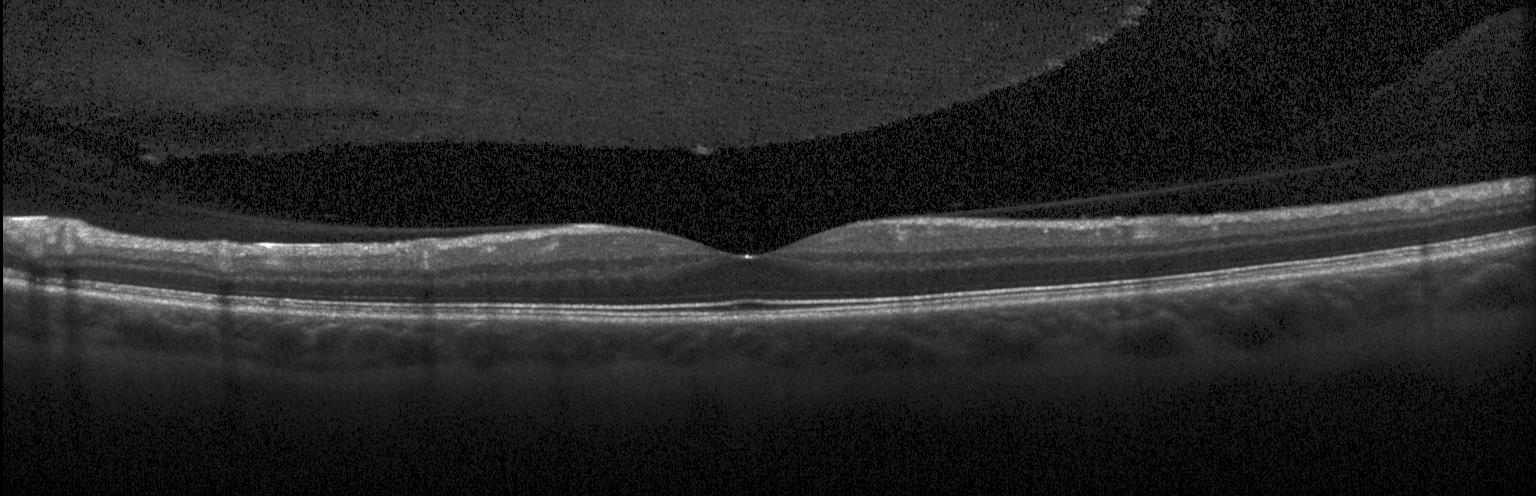 The scan shows no evidence of CNV, DME, or drusen.